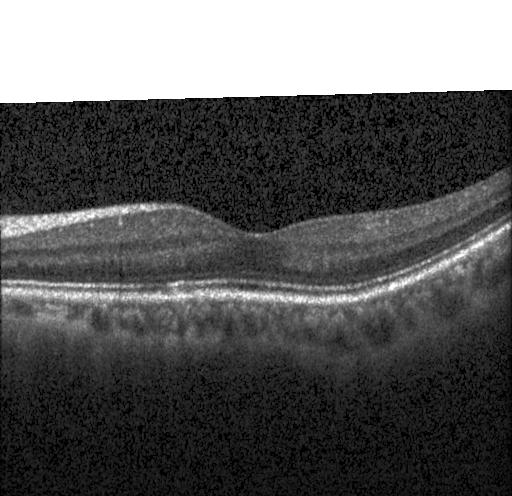

Retinal OCT B-scan. Dx: neither choroidal neovascularization, diabetic macular edema, nor drusen.